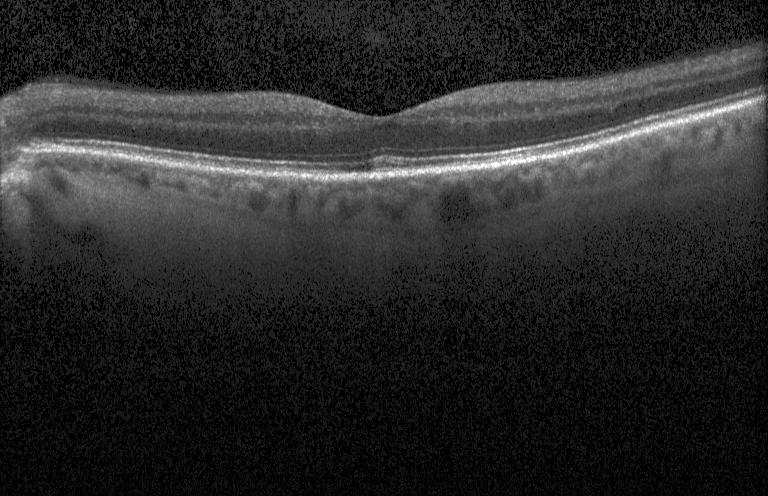

No choroidal neovascularization, diabetic macular edema, or drusen.